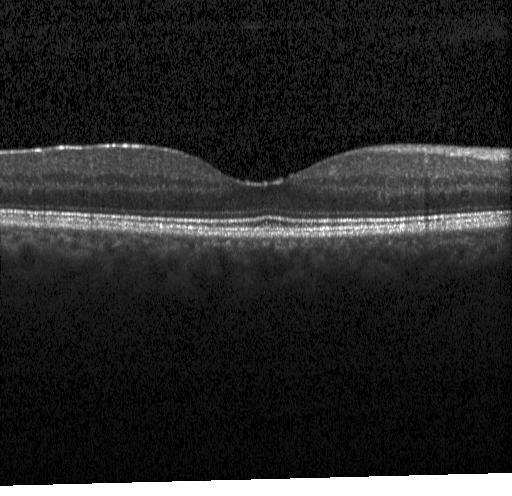

No choroidal neovascularization, diabetic macular edema, or drusen.